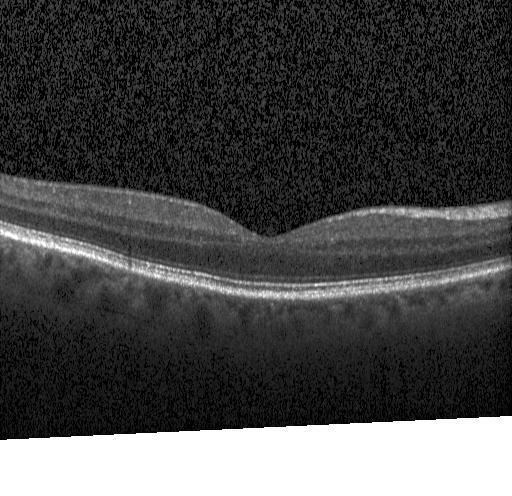 Optical coherence tomography scan. This B-scan demonstrates no evidence of choroidal neovascularization, diabetic macular edema, or drusen.